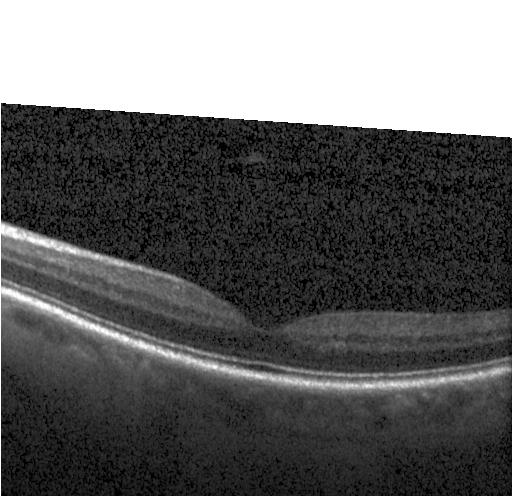

OCT finding: no choroidal neovascularization, no diabetic macular edema, and no drusen.